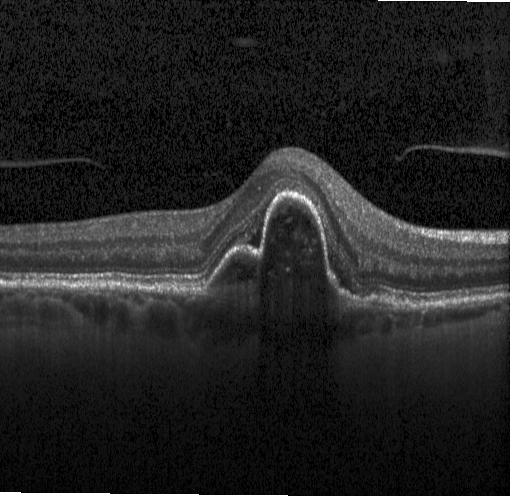 OCT line scan. Centered on the fovea. Heidelberg Spectralis.
Diagnosis: a choroidal neovascular membrane.